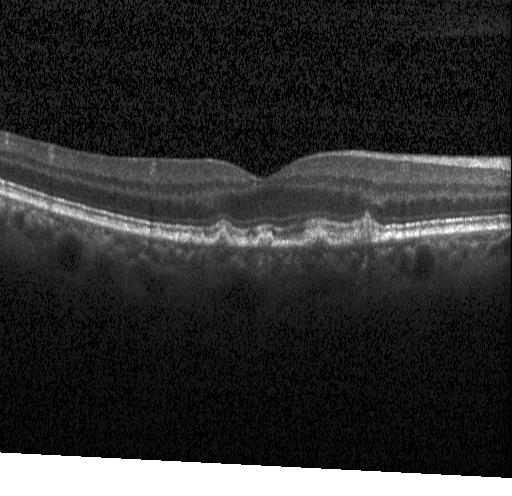
Retinal OCT cross-section.
Impression: sub-RPE drusenoid deposits.